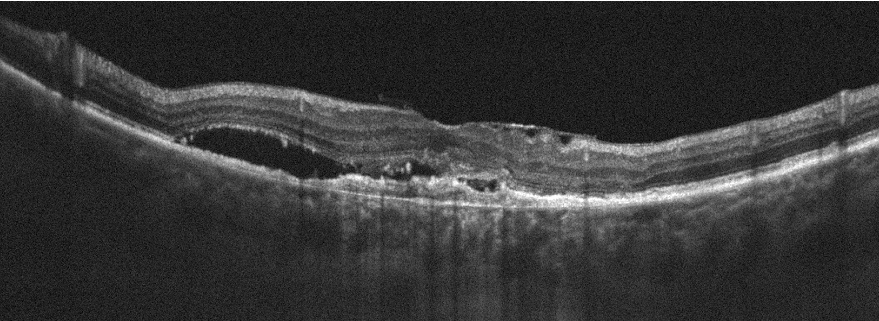
Dx: age-related macular degeneration.